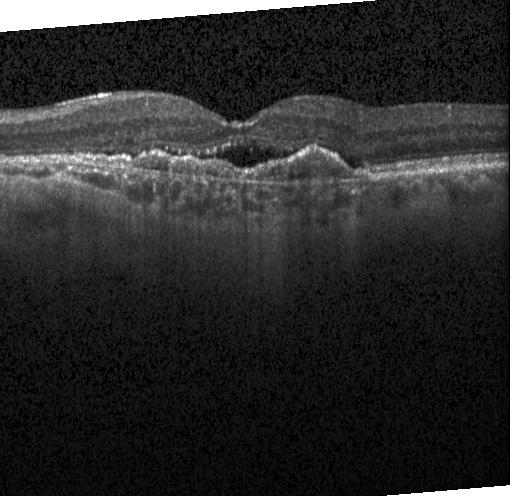
Assessment: choroidal neovascularization (CNV).